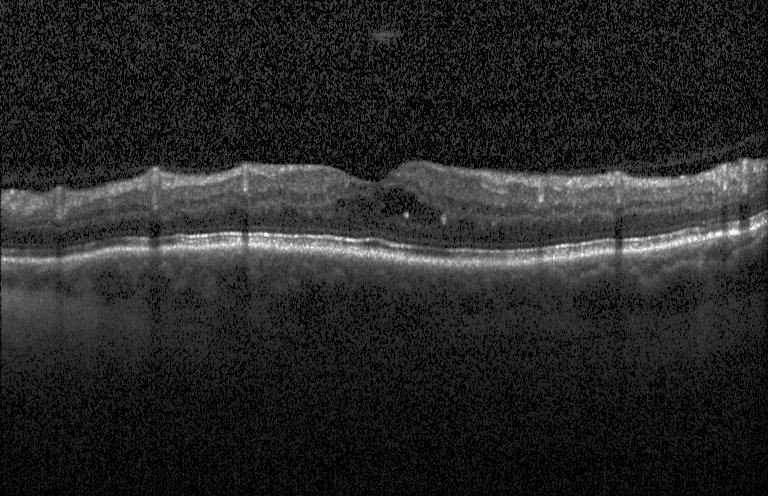 The scan shows DME.